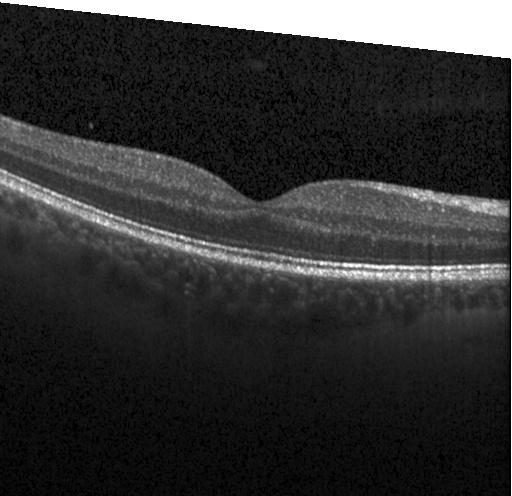

Dx: no evidence of choroidal neovascularization, diabetic macular edema, or drusen.